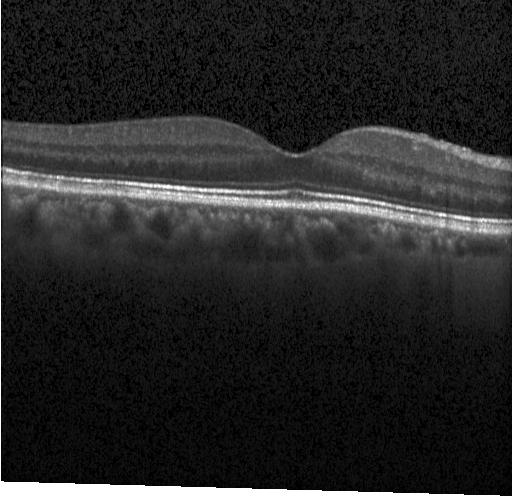 OCT B-scan, spectral-domain OCT. Diagnosis: neither choroidal neovascularization, diabetic macular edema, nor drusen.